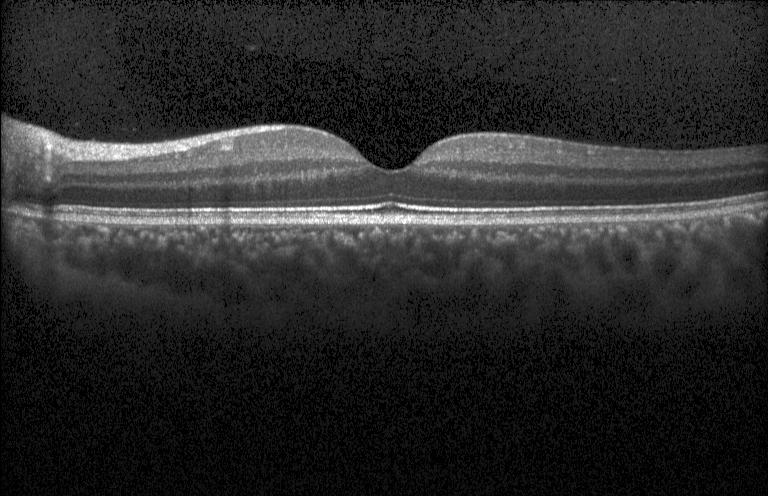
Finding: no evidence of choroidal neovascularization, diabetic macular edema, or drusen.